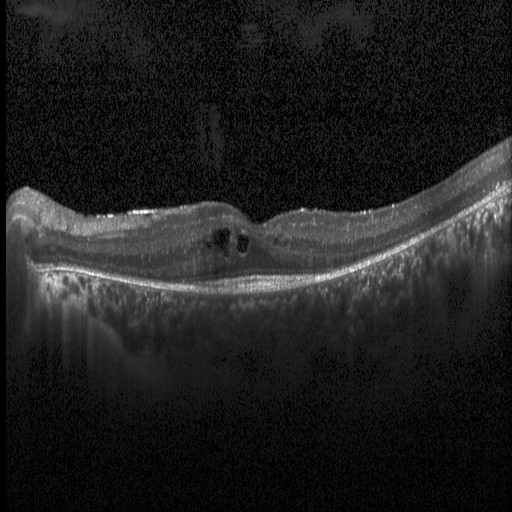

Horizontal scan through the fovea · spectral-domain optical coherence tomography · optical coherence tomography B-scan · Heidelberg Spectralis OCT system — Diabetic macular edema (DME).